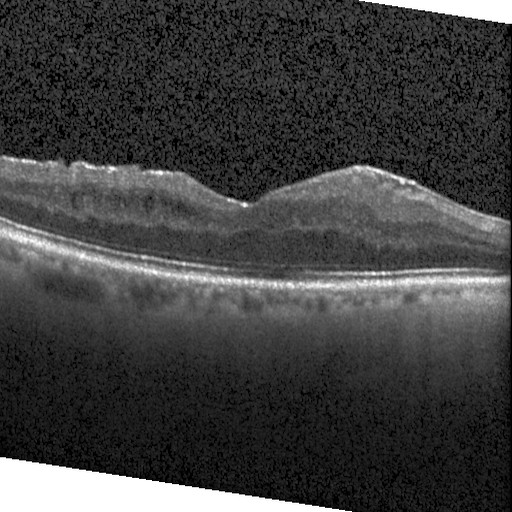

Macular OCT: diabetic macular edema (DME).